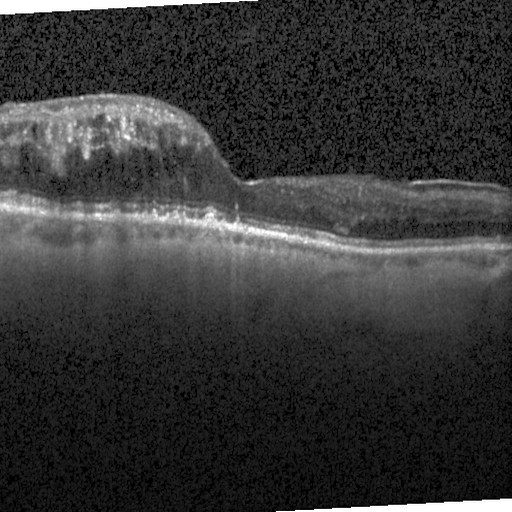
OCT B-scan showing diabetic macular edema (DME).